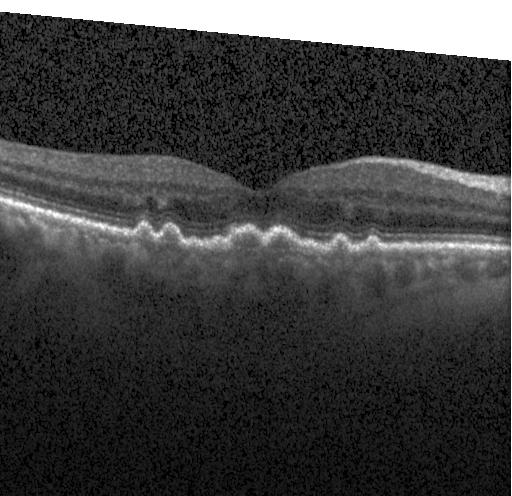

Impression: drusen.